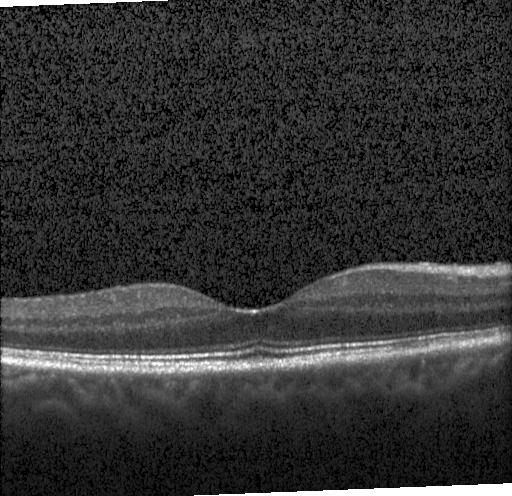 SD-OCT. Macular scan. OCT B-scan. Heidelberg Spectralis OCT system.
Macular OCT: neither choroidal neovascularization, diabetic macular edema, nor drusen.